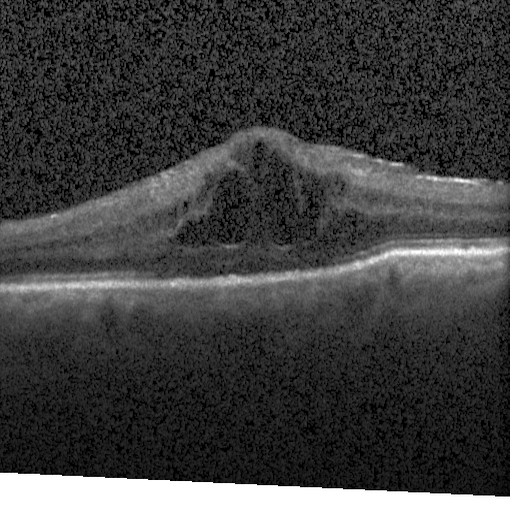

Finding: diabetic macular edema.